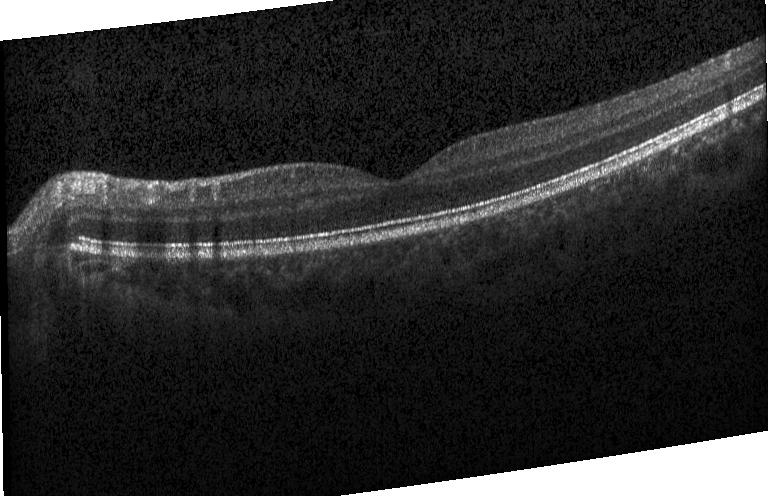

Horizontal scan through the fovea · retinal OCT cross-section
OCT finding: no evidence of CNV, DME, or drusen.